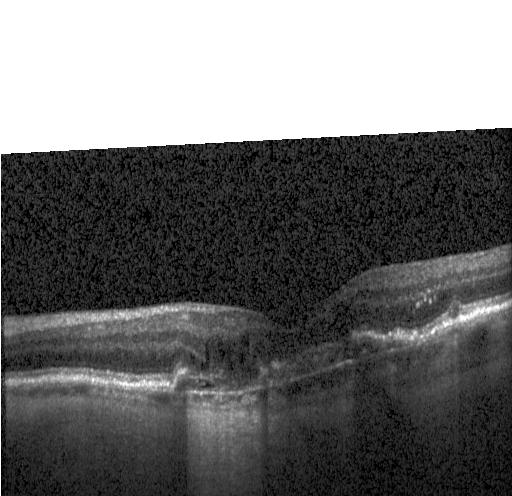 Instrument: Heidelberg Spectralis · OCT B-scan · spectral-domain optical coherence tomography.
Impression: CNV.